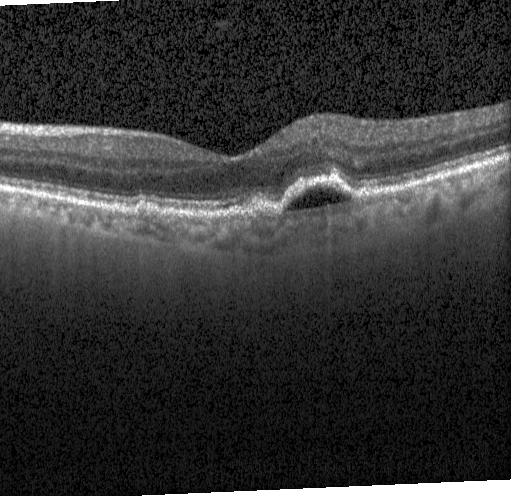

Retinal OCT cross-section showing a choroidal neovascular membrane.